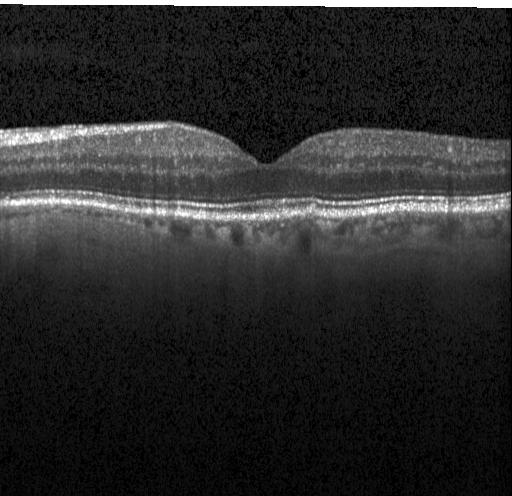
OCT line scan.
Finding: no evidence of choroidal neovascularization, diabetic macular edema, or drusen.